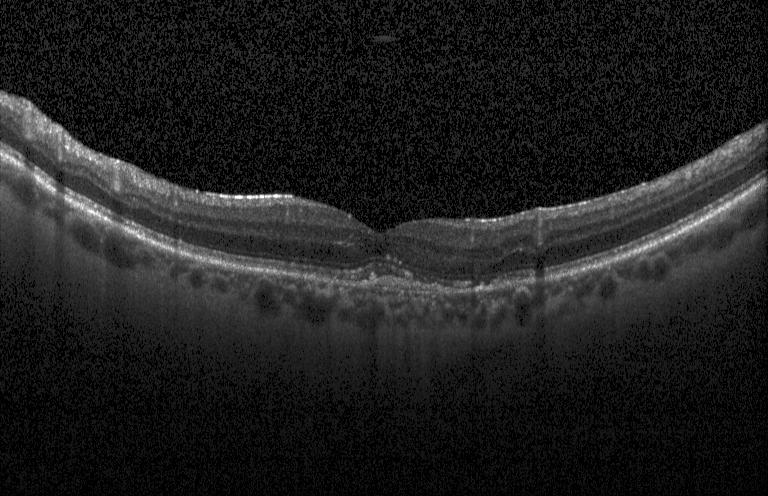

Centered on the fovea. Optical coherence tomography B-scan.
Assessment: a choroidal neovascular membrane.